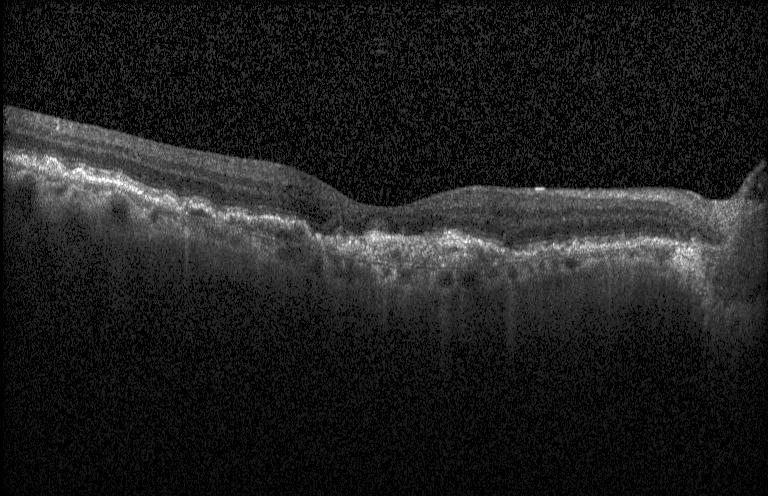

OCT B-scan showing CNV.